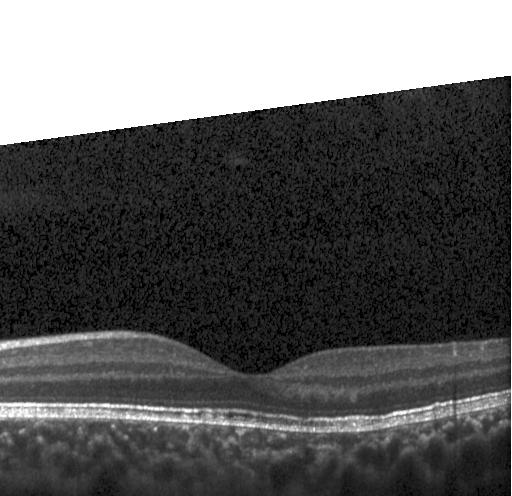
Centered on the fovea. Heidelberg Spectralis OCT system. SD-OCT. Optical coherence tomography B-scan.
Assessment: no choroidal neovascularization, no diabetic macular edema, and no drusen.